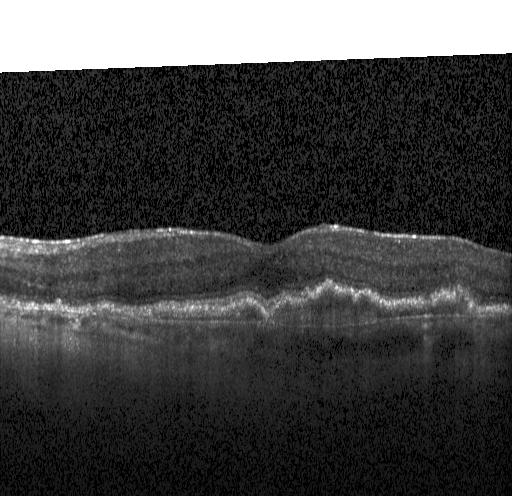
Retinal OCT cross-section.
Diagnosis: CNV.